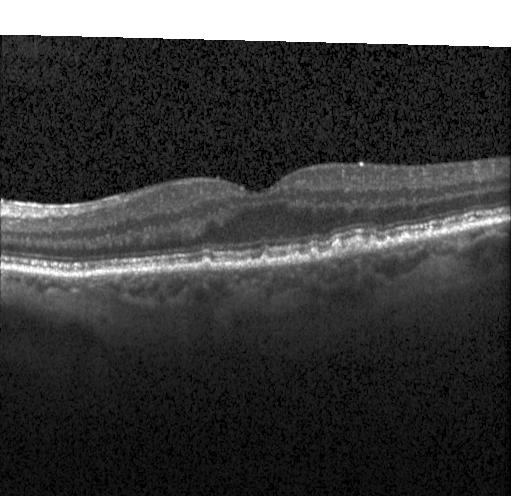 Macular OCT demonstrating sub-RPE drusenoid deposits.